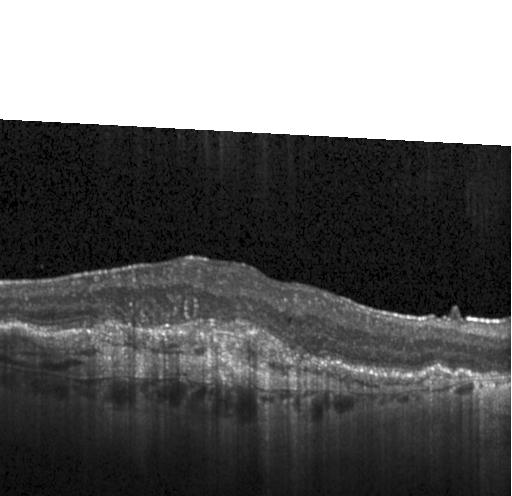

Macular OCT: choroidal neovascularization (CNV).